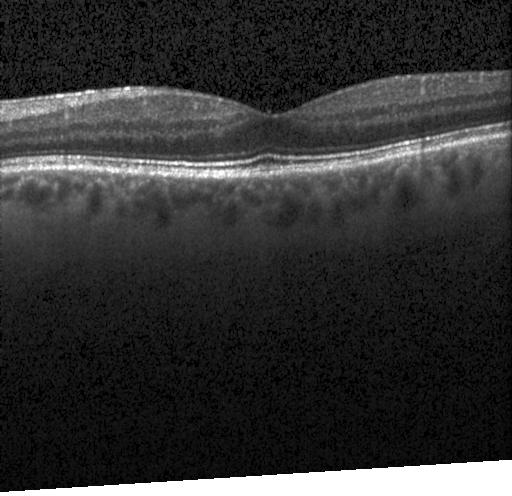

OCT B-scan showing neither choroidal neovascularization, diabetic macular edema, nor drusen.